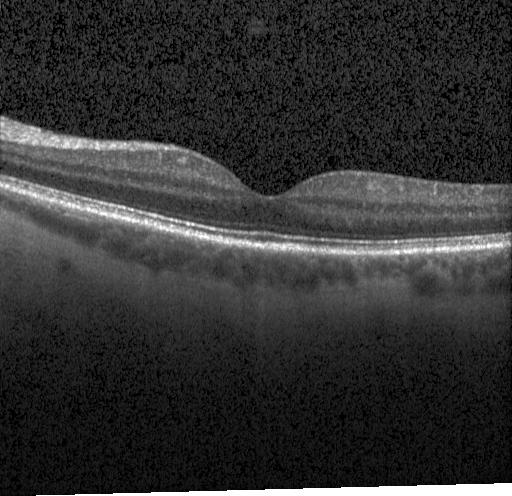 OCT line scan; through the macula; SD-OCT. No CNV, DME, or drusen.